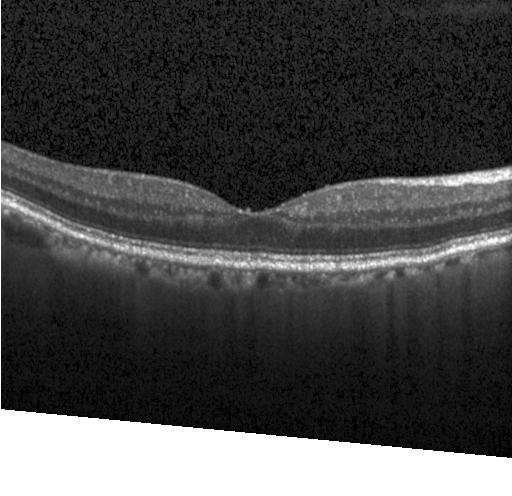 Retinal OCT cross-section. Acquired on a Heidelberg Spectralis. Horizontal scan through the fovea. OCT finding: no evidence of choroidal neovascularization, diabetic macular edema, or drusen.